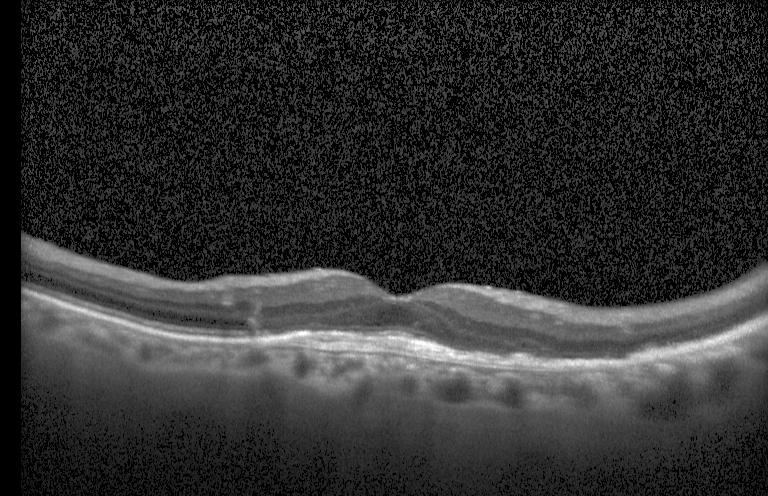
The scan shows CNV.